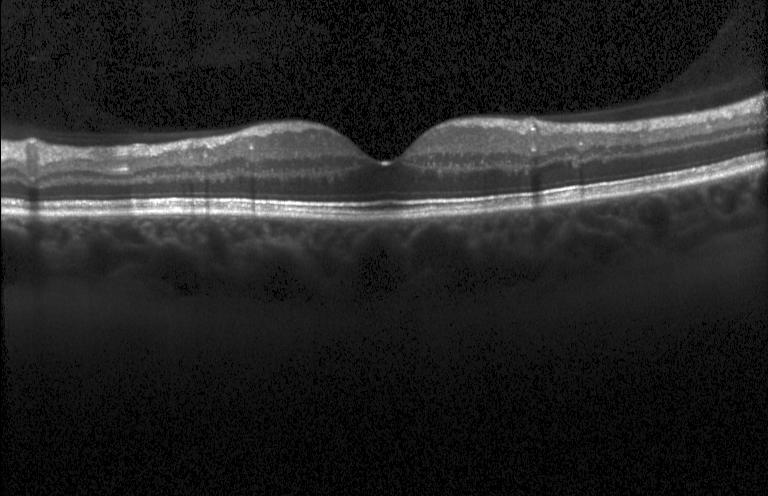 OCT line scan — Finding: no evidence of CNV, DME, or drusen.